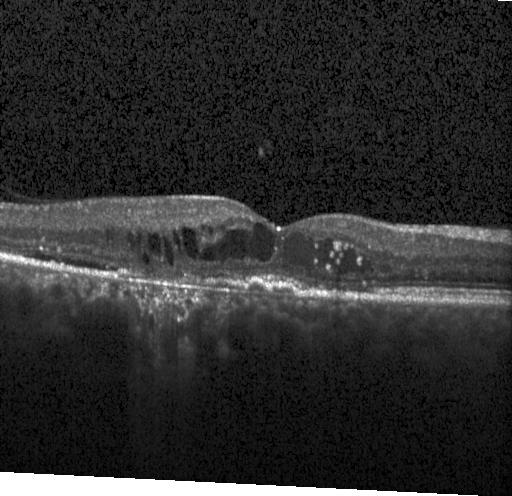
Retinal OCT cross-section · fovea-centered · Heidelberg Spectralis · spectral-domain optical coherence tomography
Impression: a choroidal neovascular membrane.